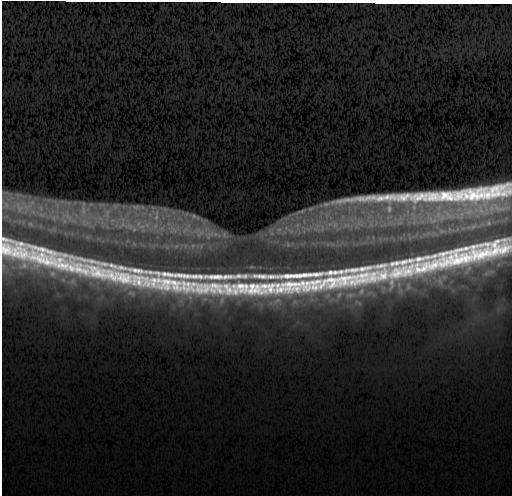

Optical coherence tomography scan, Heidelberg Spectralis OCT system, macular scan, SD-OCT. Finding: no choroidal neovascularization, no diabetic macular edema, and no drusen.